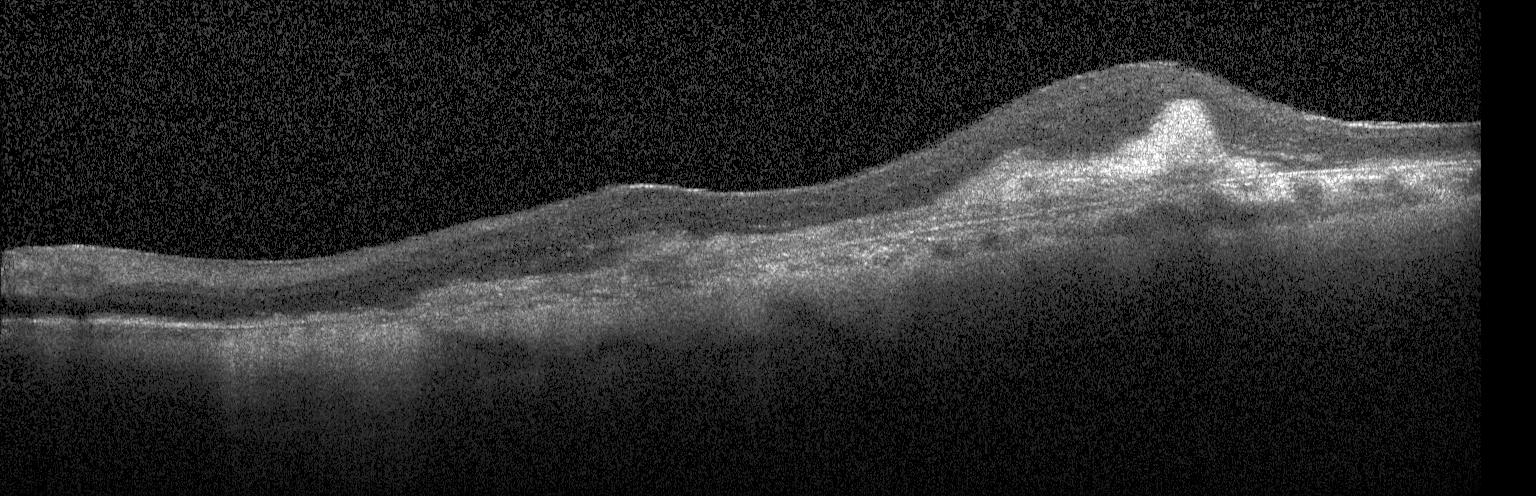

Optical coherence tomography scan. Dx: CNV.